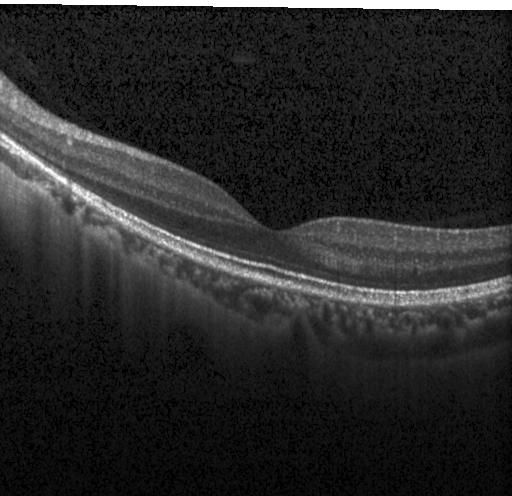
Retinal OCT B-scan. Spectral-domain OCT
Assessment: neither choroidal neovascularization, diabetic macular edema, nor drusen.